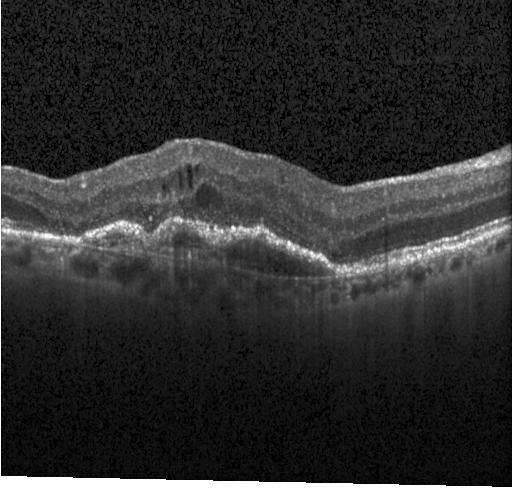
Macular OCT: a choroidal neovascular membrane.